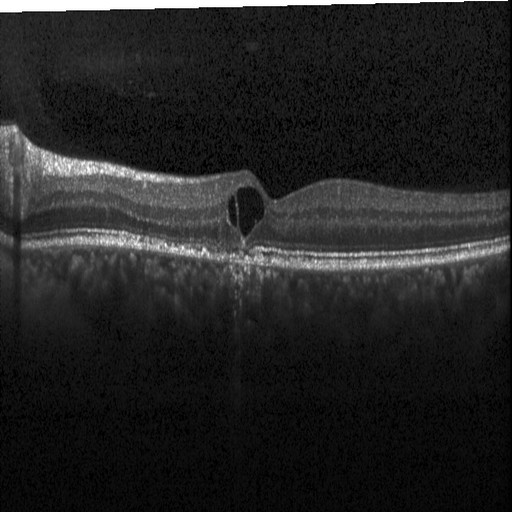

Heidelberg Spectralis · optical coherence tomography scan
This B-scan demonstrates diabetic macular edema (DME).